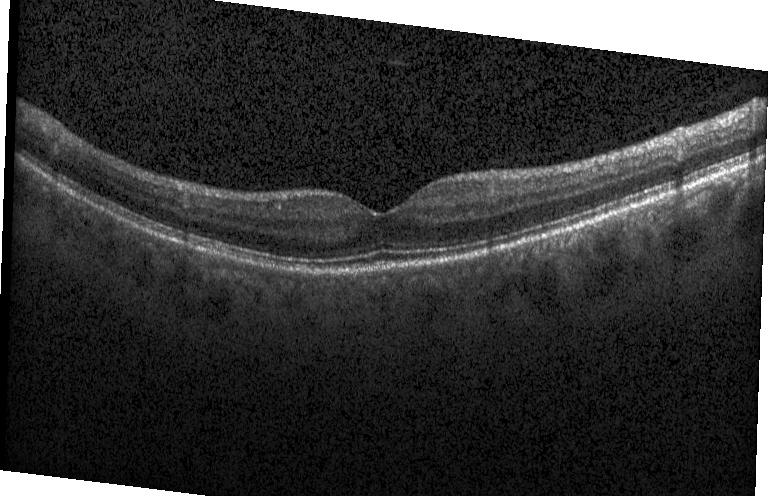

Spectral-domain OCT B-scan: no evidence of CNV, DME, or drusen.